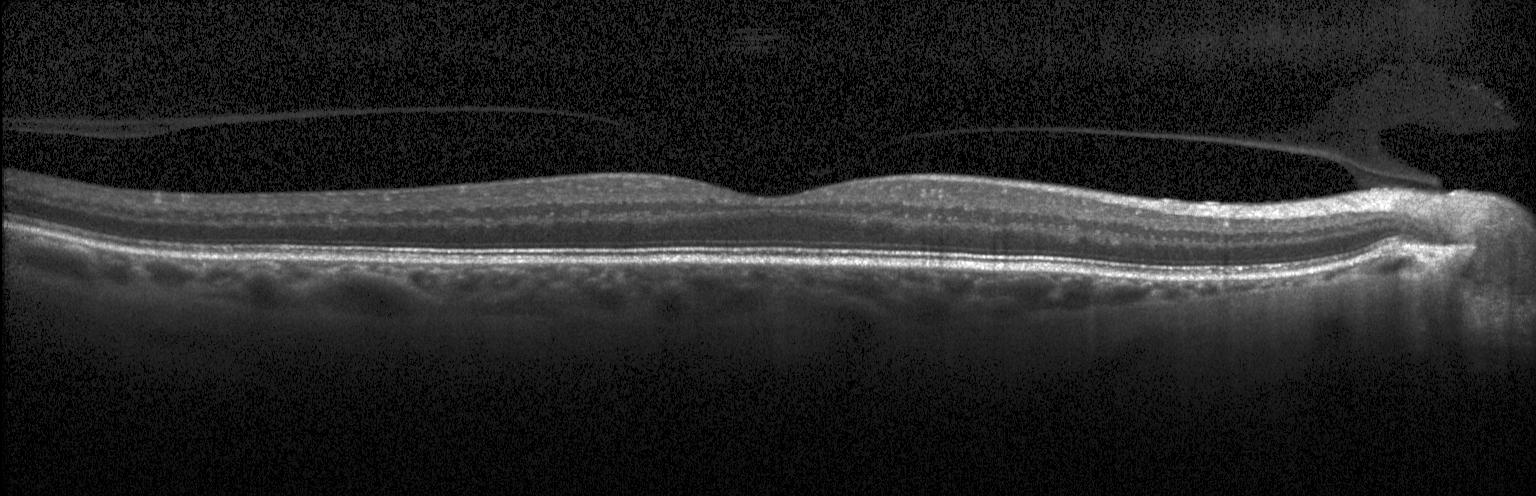
Through the macula · retinal OCT B-scan · acquired on a Heidelberg Spectralis
Assessment: no choroidal neovascularization, diabetic macular edema, or drusen.